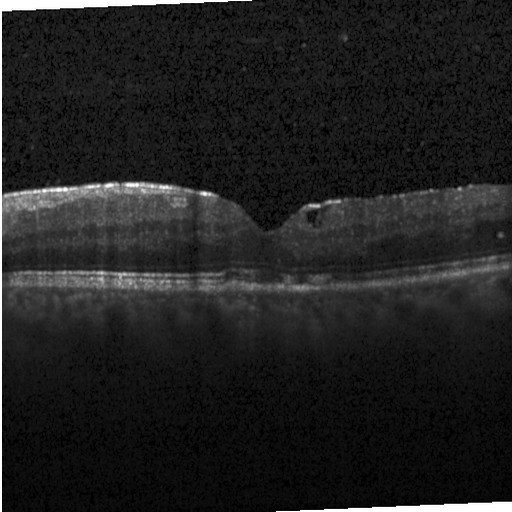

Spectral-domain optical coherence tomography. OCT B-scan.
OCT finding: diabetic macular edema.